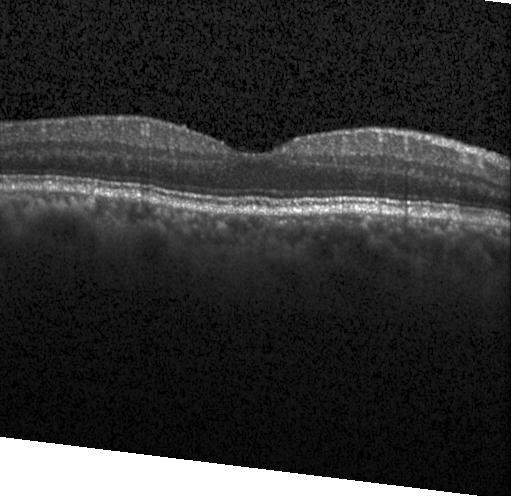

Optical coherence tomography scan
The scan shows no choroidal neovascularization, diabetic macular edema, or drusen.